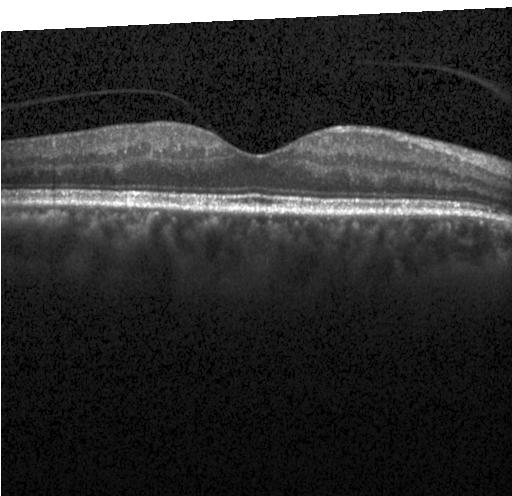 No CNV, DME, or drusen.